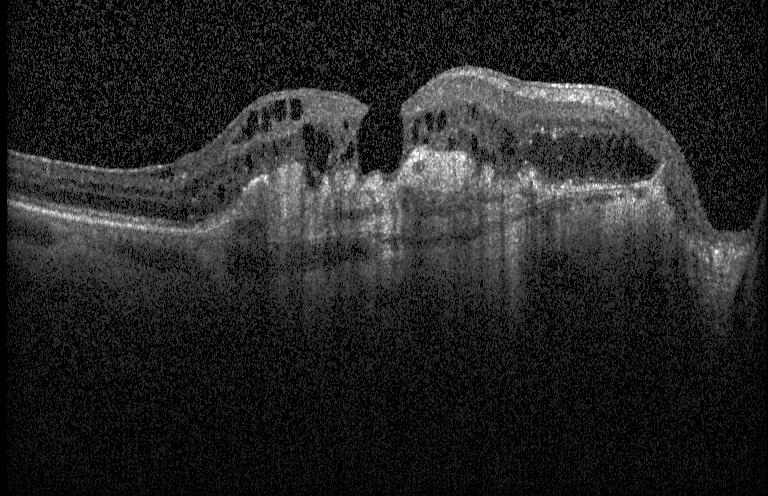 Optical coherence tomography scan. Macular OCT: choroidal neovascularization (CNV).